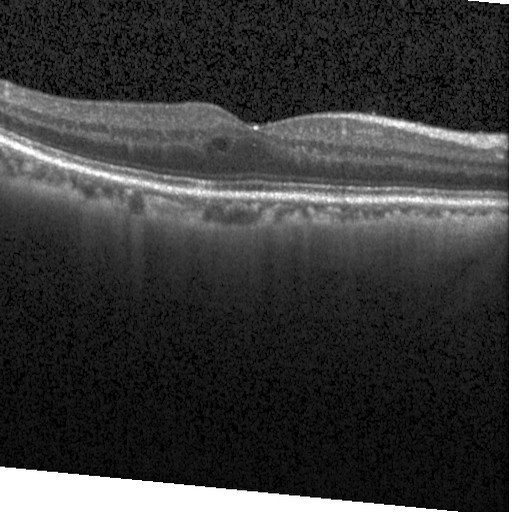

OCT line scan · centered on the fovea · SD-OCT — Impression: diabetic macular edema.